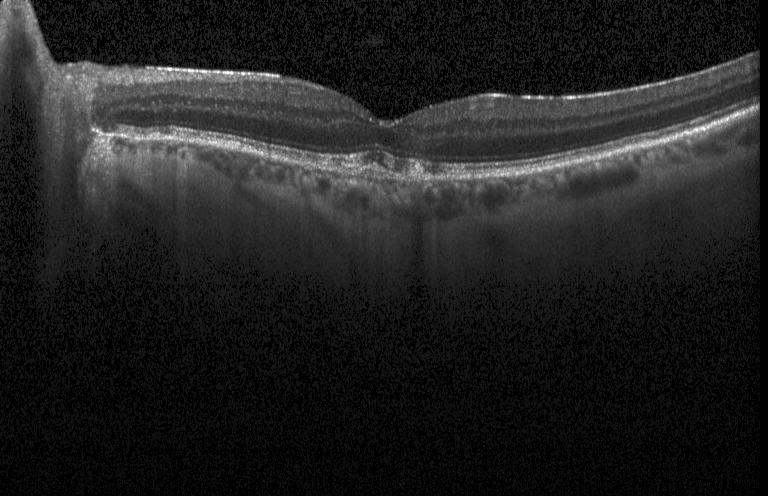
Finding: choroidal neovascularization.